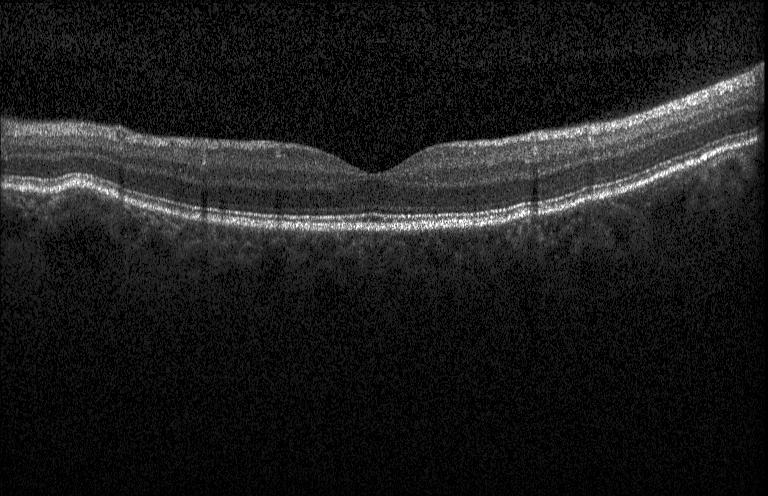

Optical coherence tomography B-scan; instrument: Heidelberg Spectralis; spectral-domain optical coherence tomography. Assessment: no choroidal neovascularization, diabetic macular edema, or drusen.